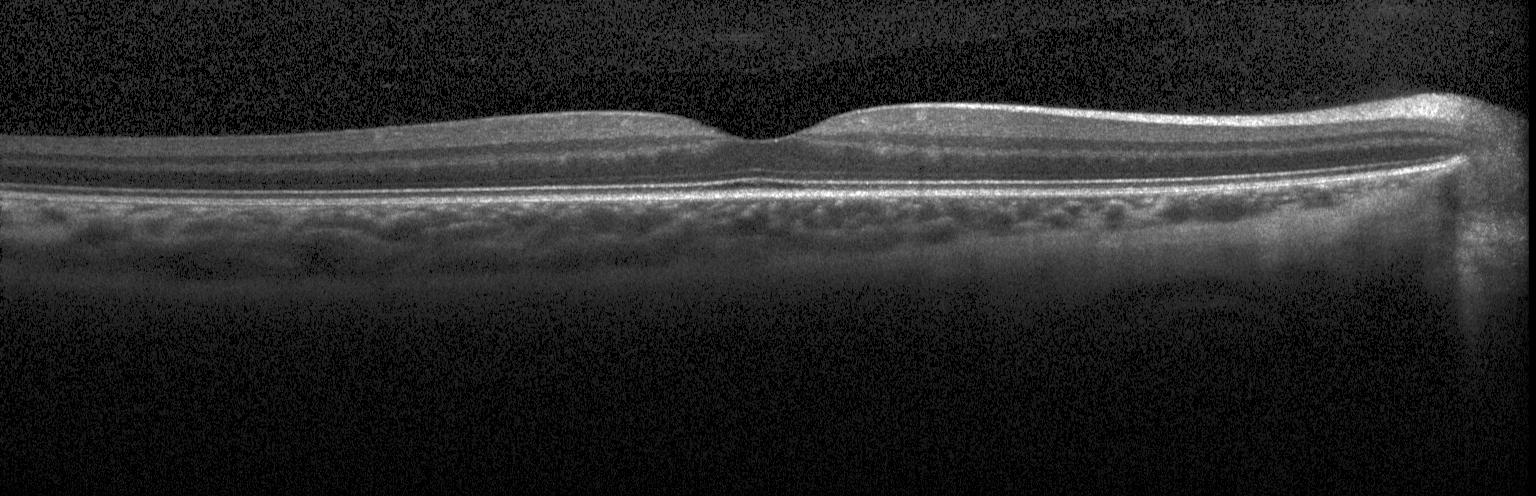 Retinal OCT cross-section
Macular OCT: no choroidal neovascularization, no diabetic macular edema, and no drusen.